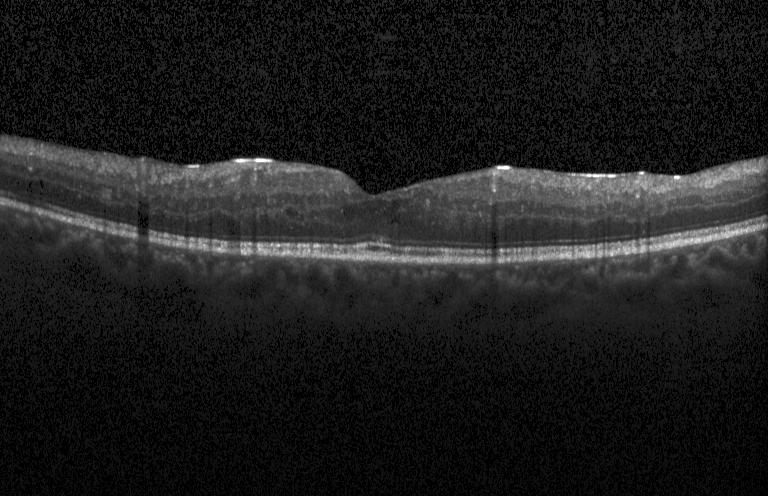

Instrument: Heidelberg Spectralis; SD-OCT; centered on the fovea; OCT line scan
OCT finding: diabetic macular edema.